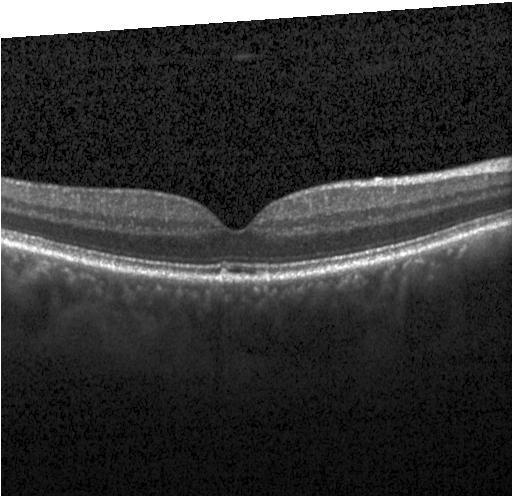
Optical coherence tomography scan, Heidelberg Spectralis OCT system
Finding: no CNV, DME, or drusen.